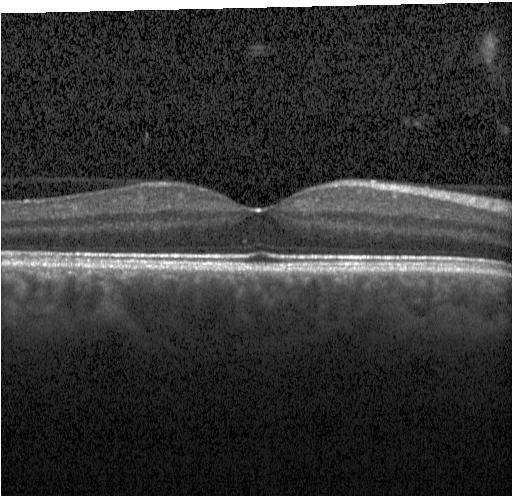 No evidence of CNV, DME, or drusen.